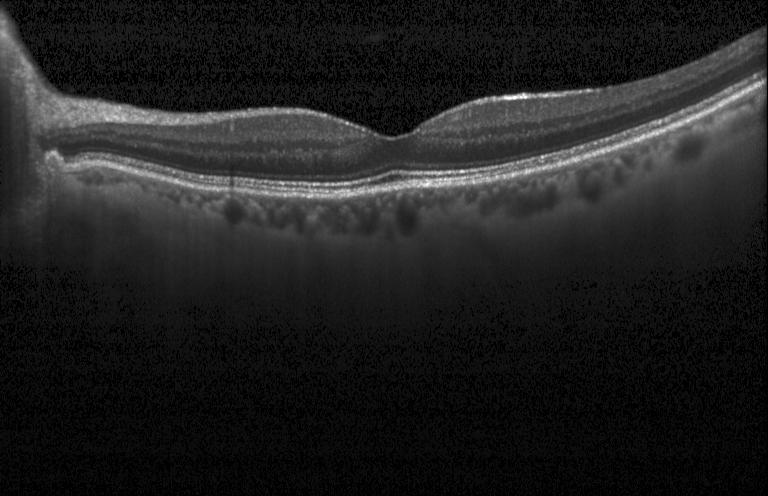
Heidelberg Spectralis, OCT line scan.
Macular OCT: no choroidal neovascularization, no diabetic macular edema, and no drusen.